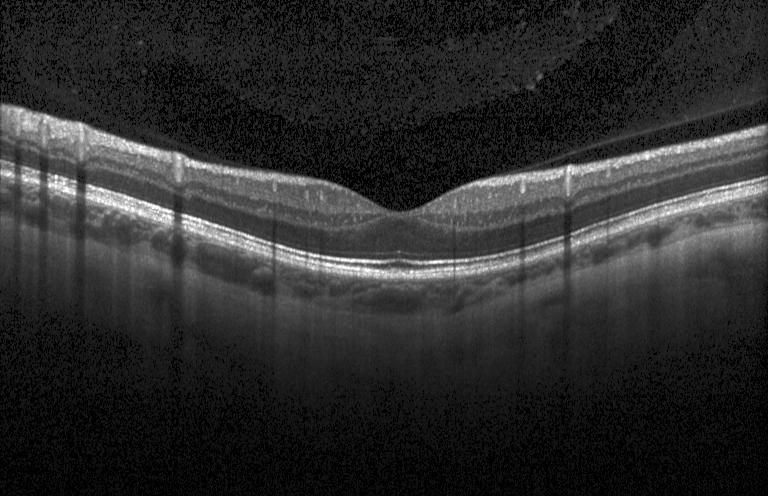 Dx: neither choroidal neovascularization, diabetic macular edema, nor drusen.